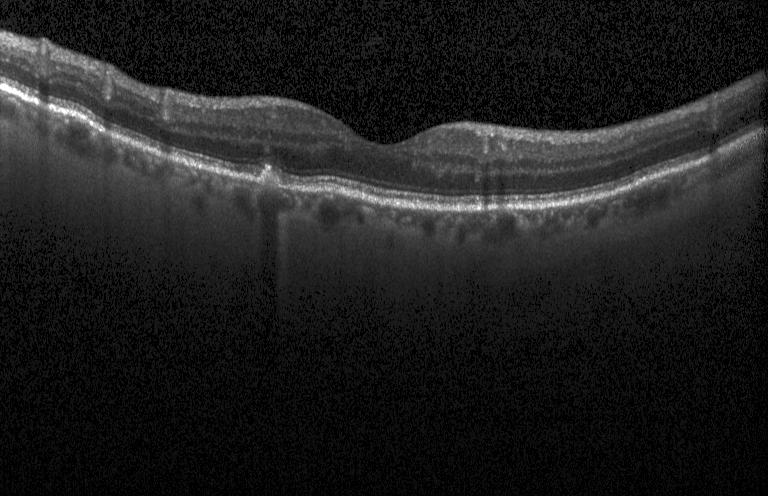

Impression: sub-RPE drusenoid deposits.